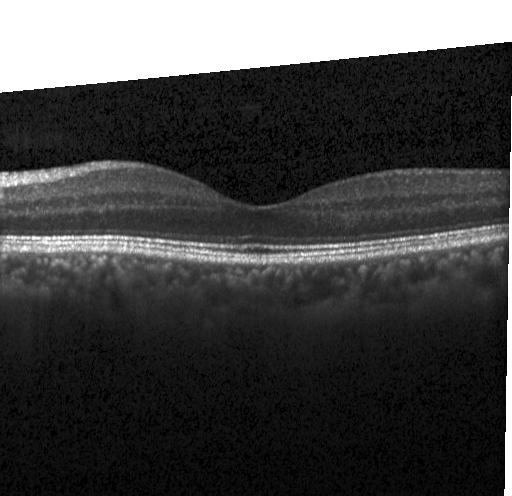

Optical coherence tomography B-scan.
This B-scan demonstrates neither choroidal neovascularization, diabetic macular edema, nor drusen.